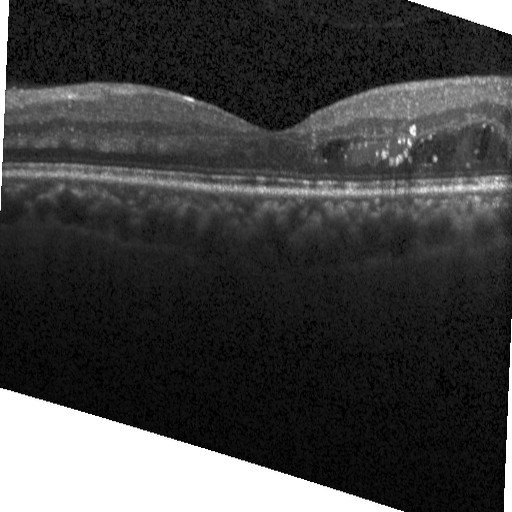
Diagnosis: DME.